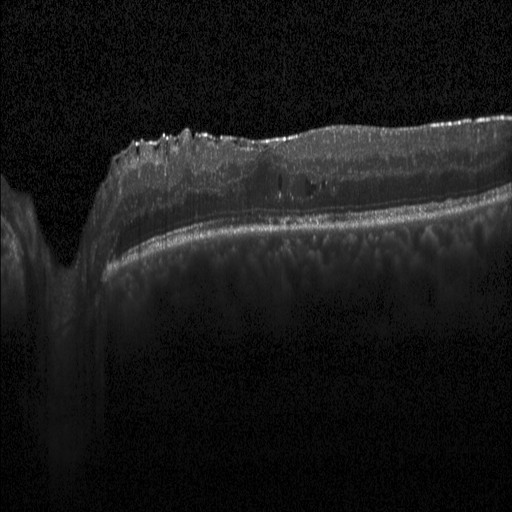 Dx: DME.